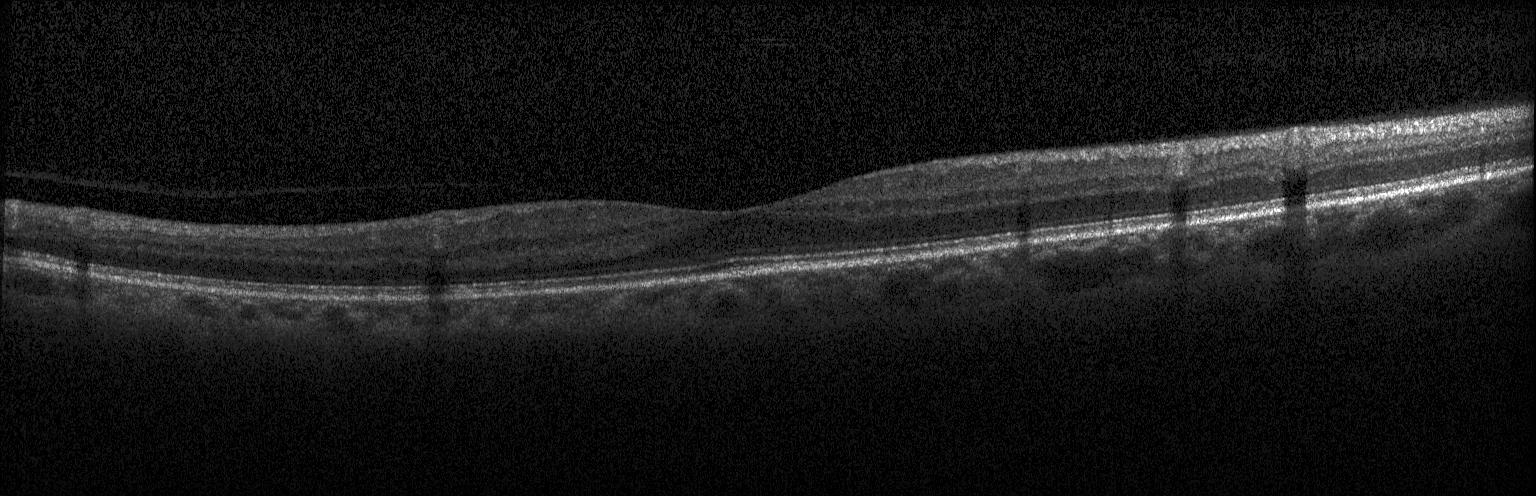 Heidelberg Spectralis OCT system · OCT line scan
Neither choroidal neovascularization, diabetic macular edema, nor drusen.